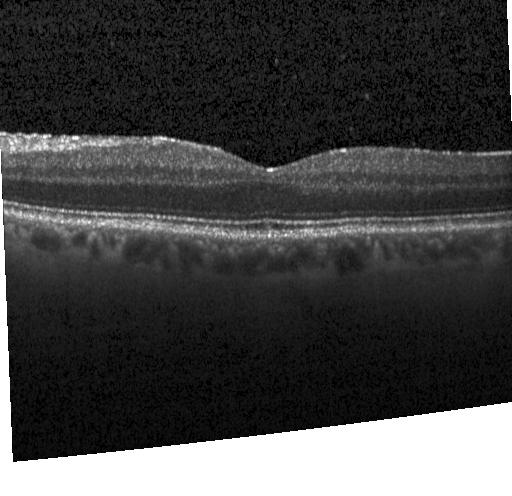

Through the macula, OCT line scan — Diagnosis: no evidence of choroidal neovascularization, diabetic macular edema, or drusen.